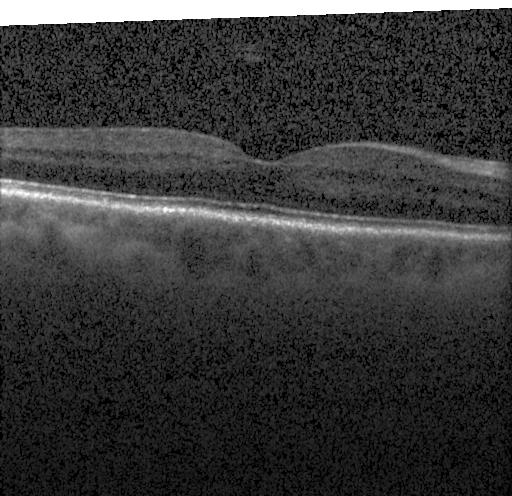
OCT finding: neither choroidal neovascularization, diabetic macular edema, nor drusen.